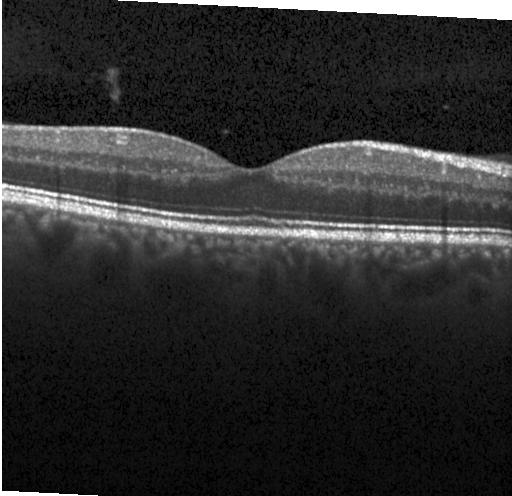

No CNV, DME, or drusen.